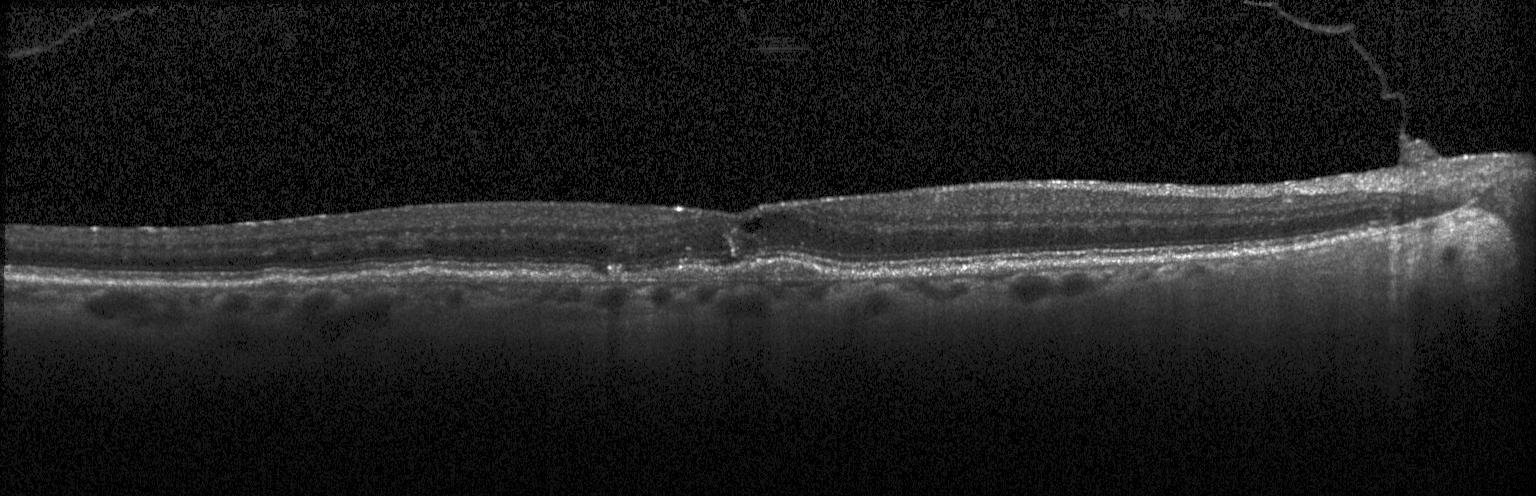

Retinal OCT cross-section
Impression: choroidal neovascularization.